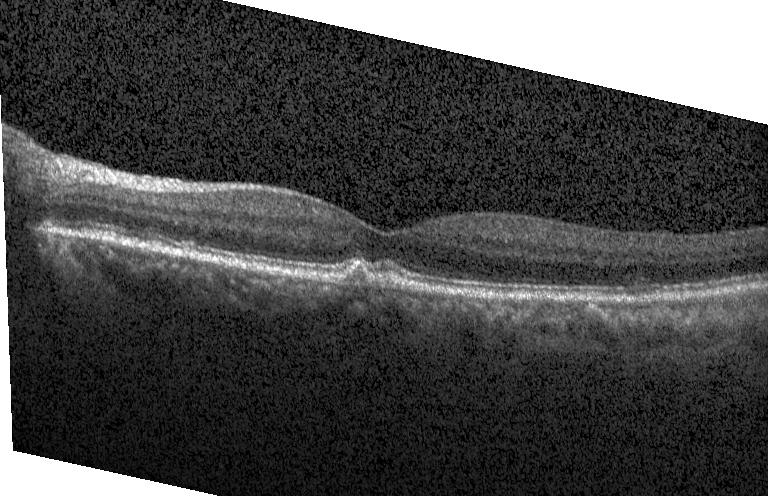

Finding: multiple drusen.